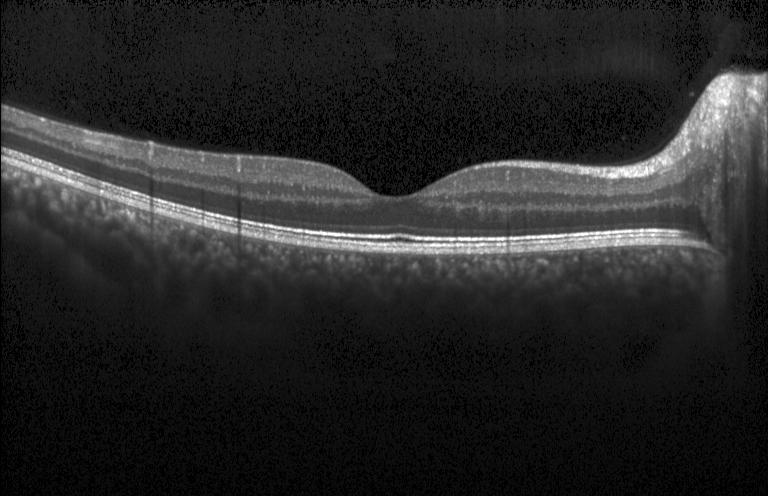 Acquired on a Heidelberg Spectralis, retinal OCT B-scan — No choroidal neovascularization, no diabetic macular edema, and no drusen.